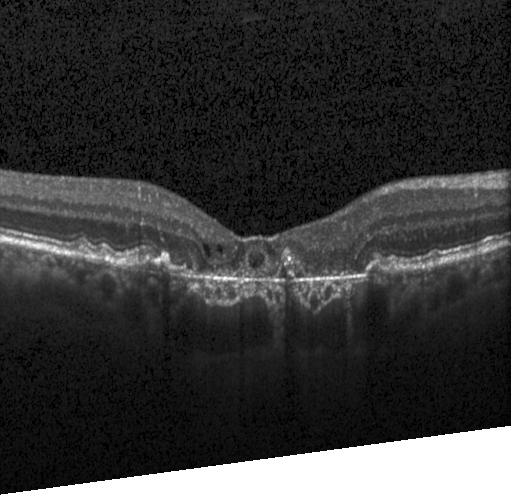

The scan shows choroidal neovascularization.